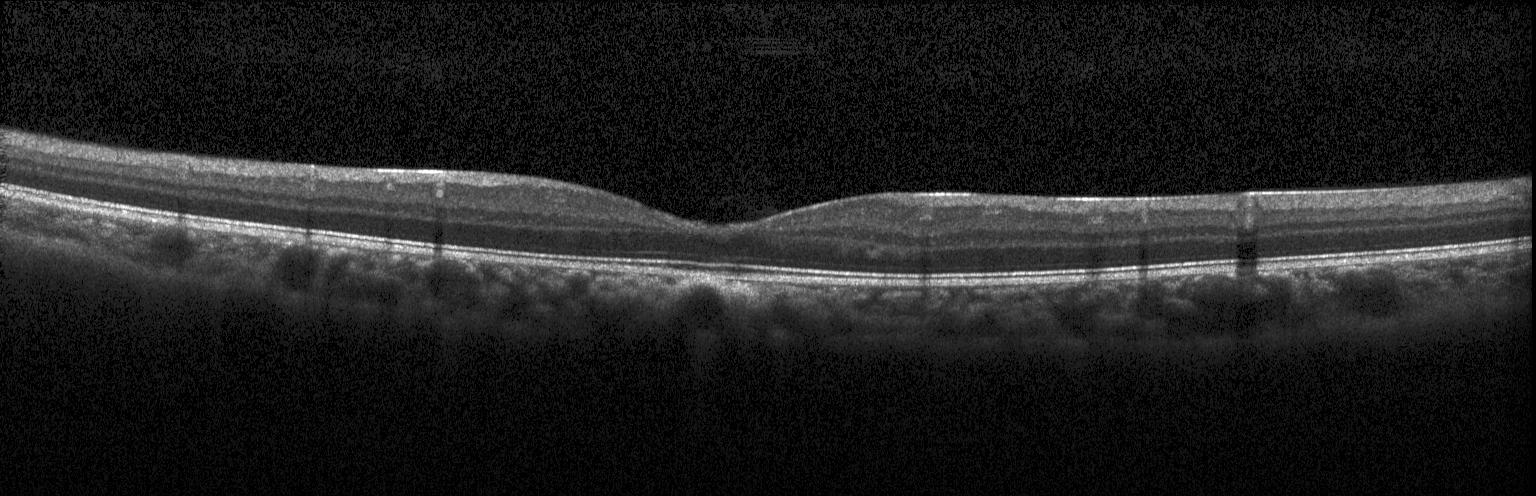

Retinal OCT cross-section.
The scan shows no choroidal neovascularization, no diabetic macular edema, and no drusen.